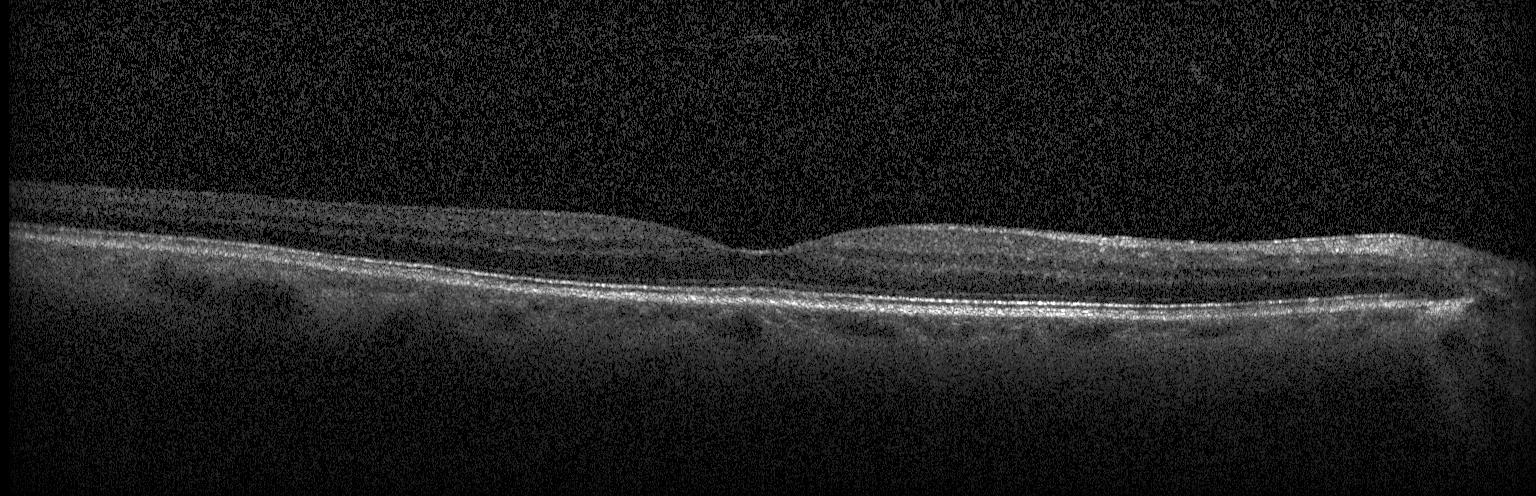 No CNV, no DME, and no drusen.